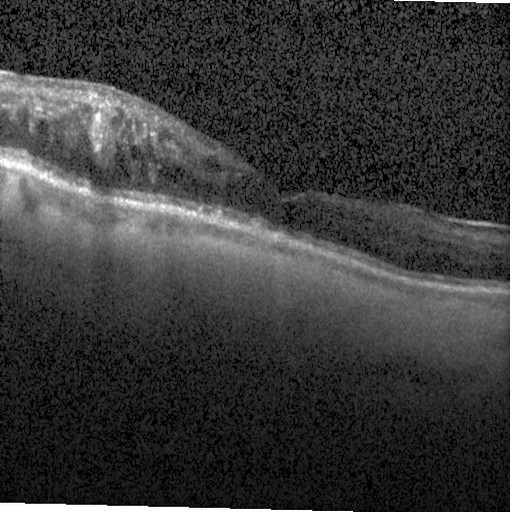
Assessment: diabetic macular edema (DME).